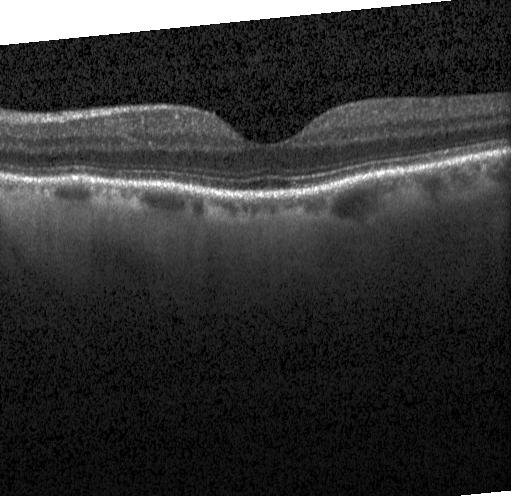
Retinal OCT cross-section showing neither CNV, DME, nor drusen.